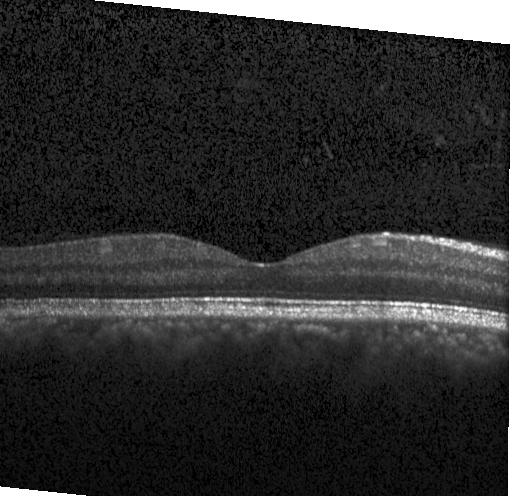 Through the macula · optical coherence tomography scan · SD-OCT · Heidelberg Spectralis OCT system.
This B-scan demonstrates no evidence of choroidal neovascularization, diabetic macular edema, or drusen.